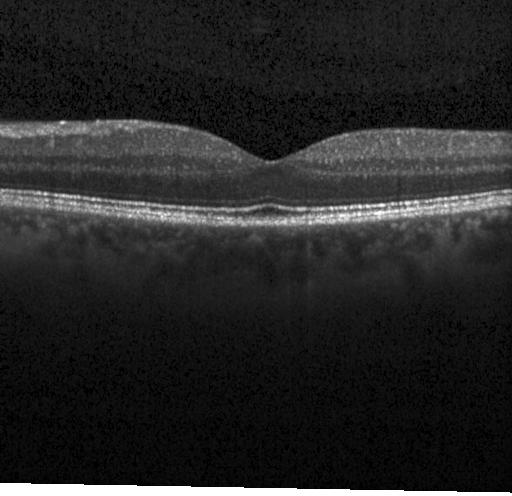

OCT line scan.
Diagnosis: no CNV, DME, or drusen.